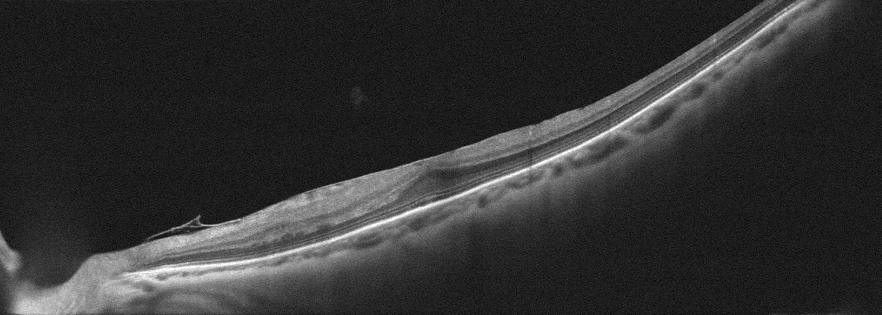
The scan shows epiretinal membrane.